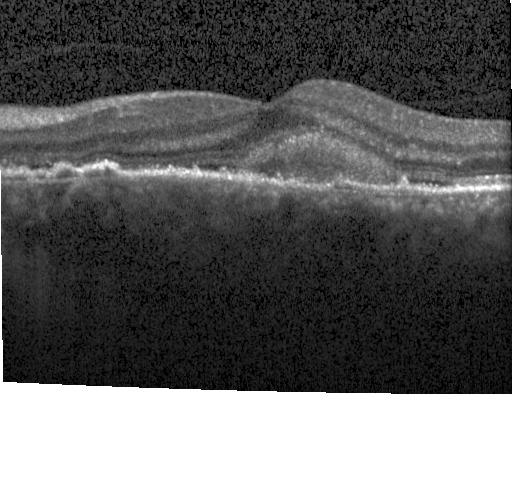
Retinal OCT B-scan — Finding: a choroidal neovascular membrane.